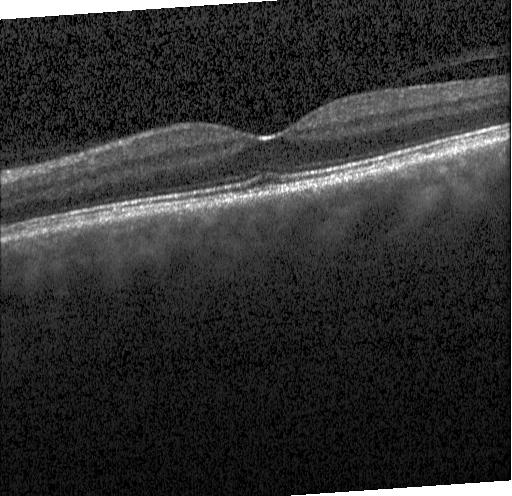
Heidelberg Spectralis OCT system; centered on the fovea; optical coherence tomography B-scan. Assessment: no evidence of choroidal neovascularization, diabetic macular edema, or drusen.